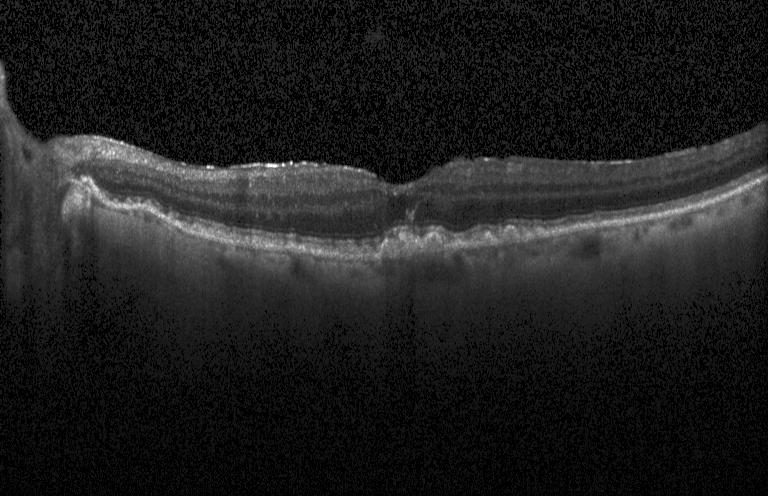 Impression: sub-RPE drusenoid deposits.